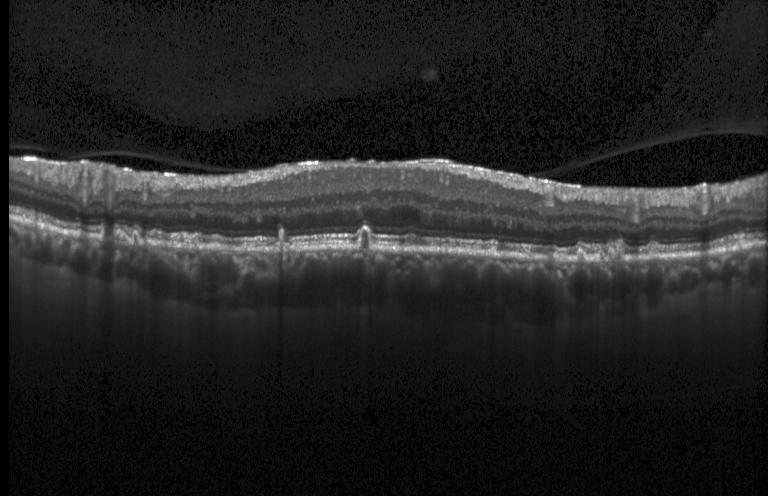
Optical coherence tomography B-scan · spectral-domain OCT.
This B-scan demonstrates drusen.